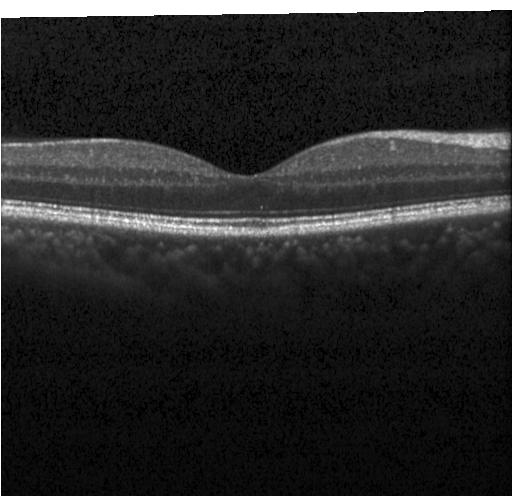

Macular OCT: no choroidal neovascularization, no diabetic macular edema, and no drusen.